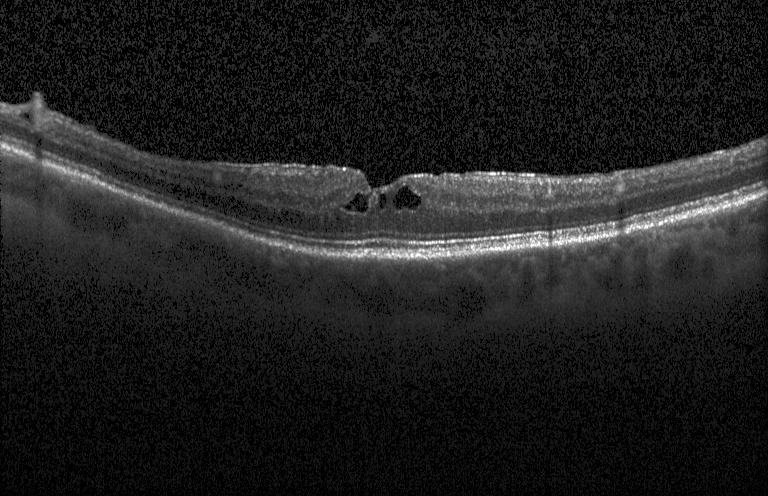 Optical coherence tomography scan
Finding: diabetic macular edema (DME).